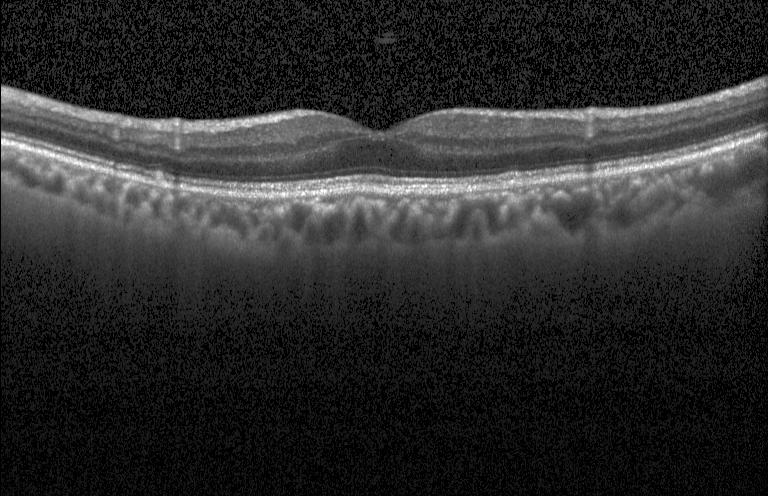
Optical coherence tomography B-scan. Dx: no choroidal neovascularization, no diabetic macular edema, and no drusen.